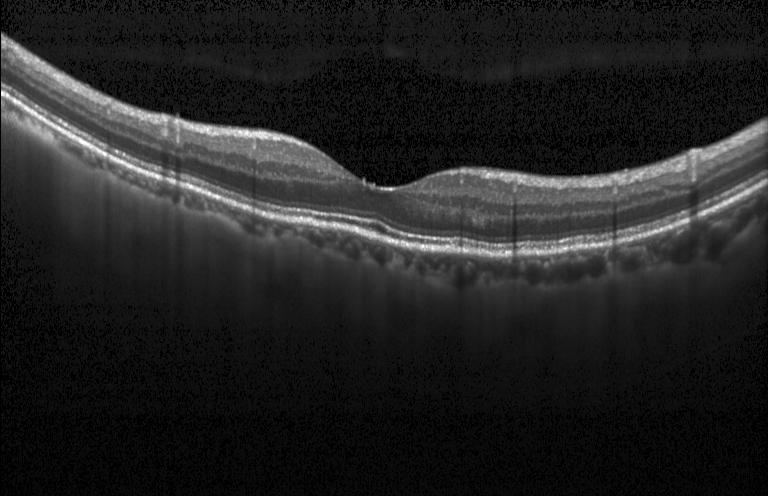

Macular OCT: no evidence of choroidal neovascularization, diabetic macular edema, or drusen.